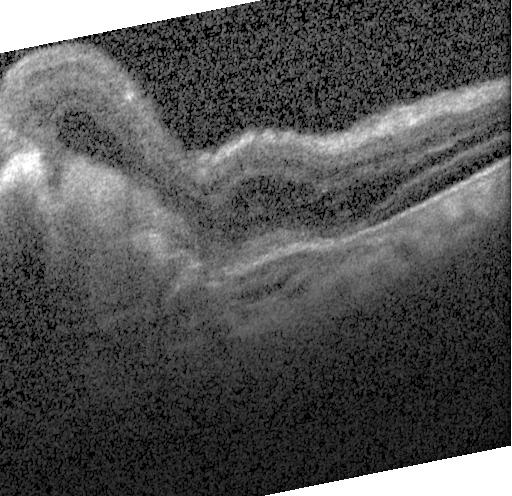

Retinal OCT cross-section showing a choroidal neovascular membrane.